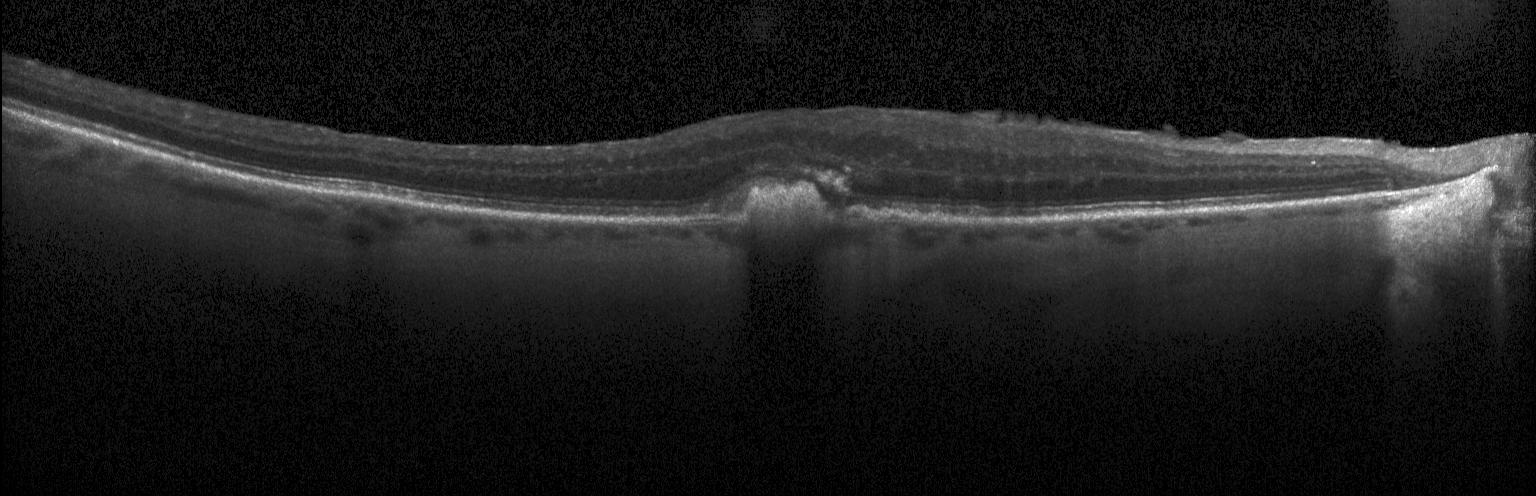
OCT finding: a choroidal neovascular membrane.